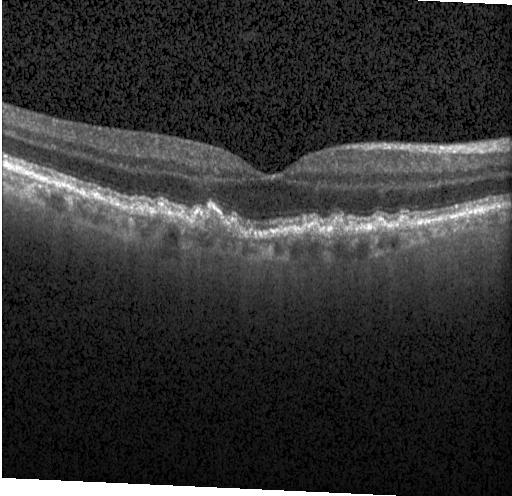
OCT line scan; fovea-centered; Heidelberg Spectralis; spectral-domain OCT.
Finding: drusen.